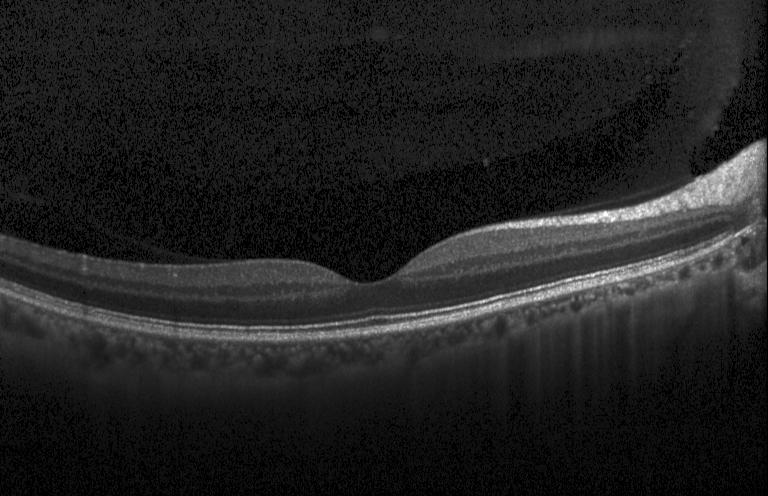

Finding: no choroidal neovascularization, diabetic macular edema, or drusen.